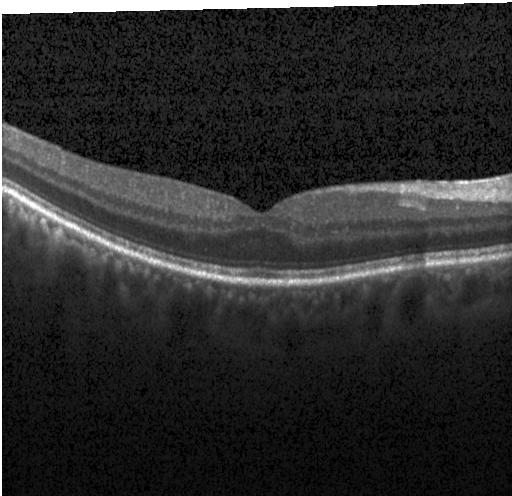

Through the macula; retinal OCT cross-section — The scan shows no choroidal neovascularization, diabetic macular edema, or drusen.